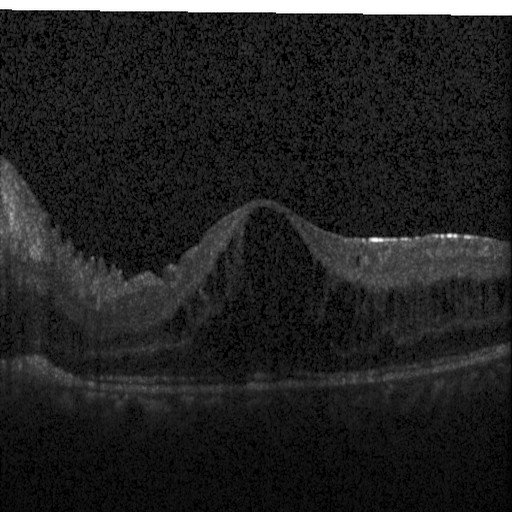 Optical coherence tomography B-scan; spectral-domain OCT; centered on the fovea; Heidelberg Spectralis
This B-scan demonstrates diabetic macular edema (DME).